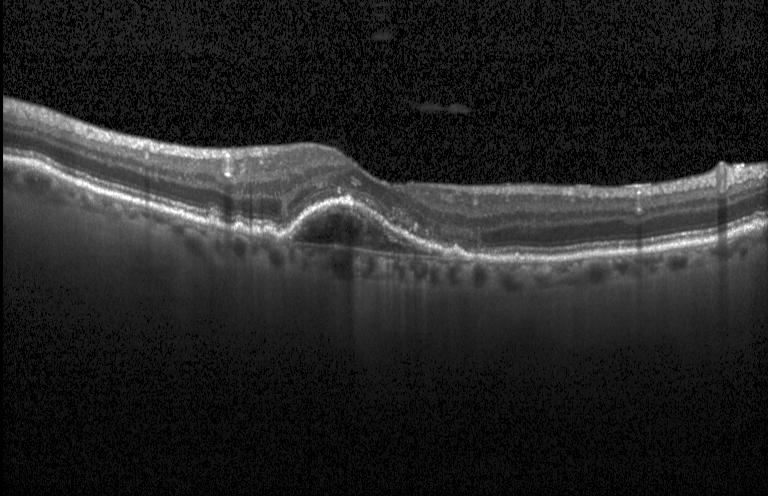 Retinal OCT cross-section, through the macula, SD-OCT
Dx: a choroidal neovascular membrane.